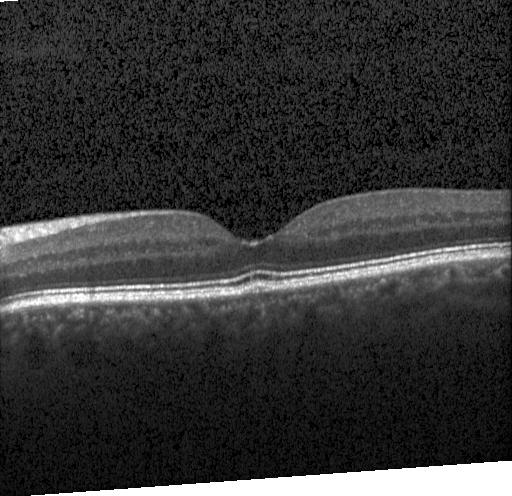

Retinal OCT B-scan. Spectral-domain OCT
The scan shows no choroidal neovascularization, diabetic macular edema, or drusen.